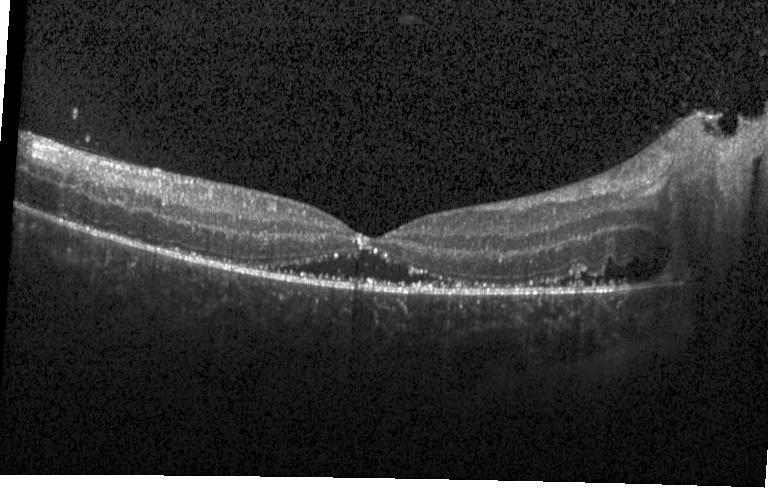

Retinal OCT cross-section.
This B-scan demonstrates choroidal neovascularization (CNV).